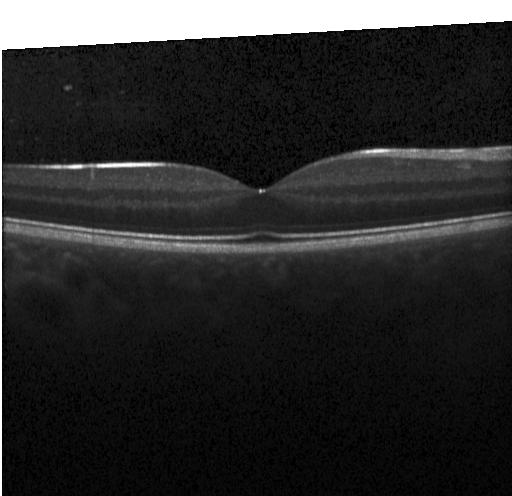
Retinal OCT B-scan. Diagnosis: no choroidal neovascularization, no diabetic macular edema, and no drusen.